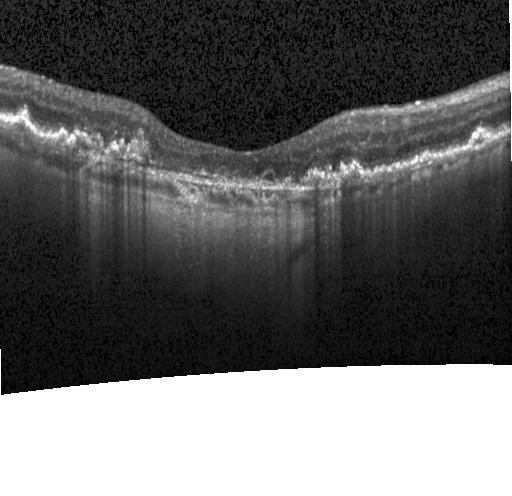 OCT B-scan — Assessment: choroidal neovascularization.